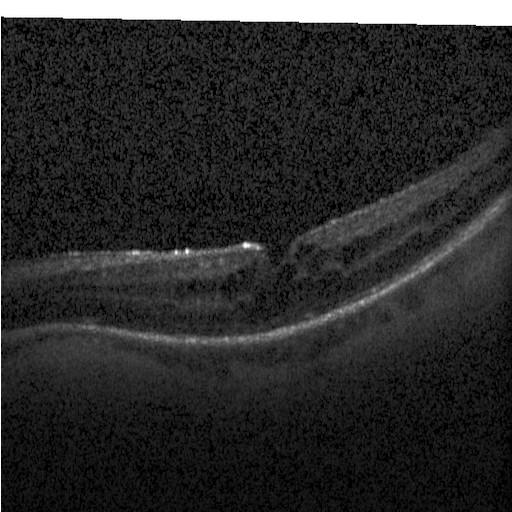
Horizontal scan through the fovea; acquired on a Heidelberg Spectralis; OCT B-scan; spectral-domain optical coherence tomography
OCT finding: DME.